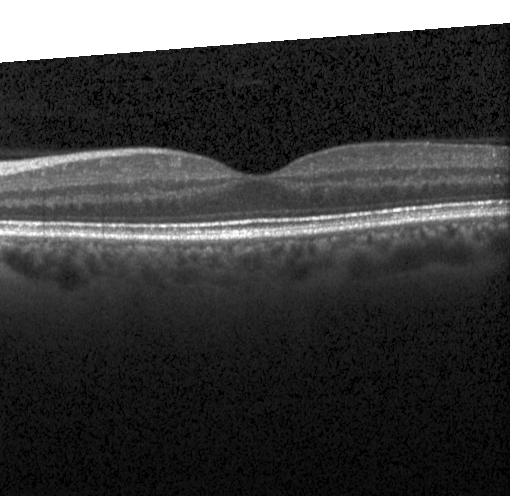 Retinal OCT B-scan
Finding: neither choroidal neovascularization, diabetic macular edema, nor drusen.